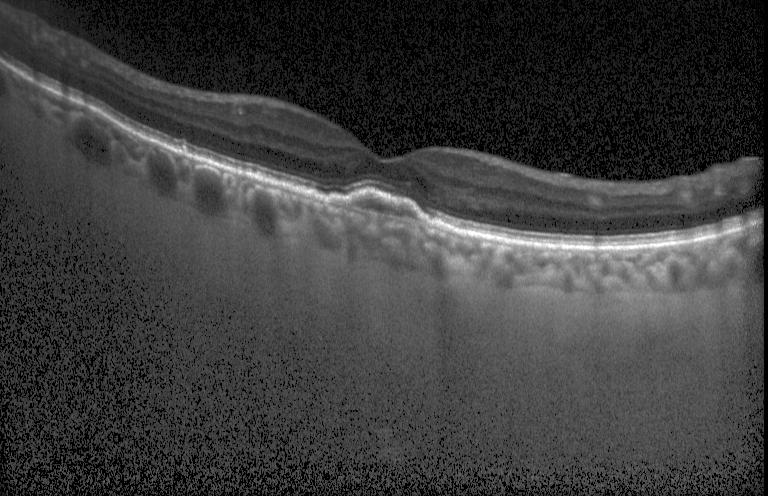
OCT B-scan showing CNV.